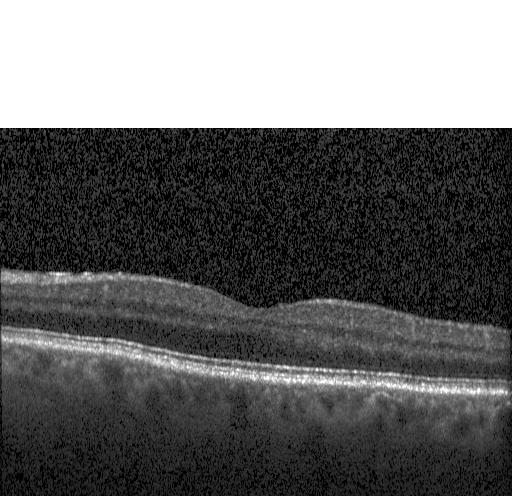 Assessment: no choroidal neovascularization, no diabetic macular edema, and no drusen.